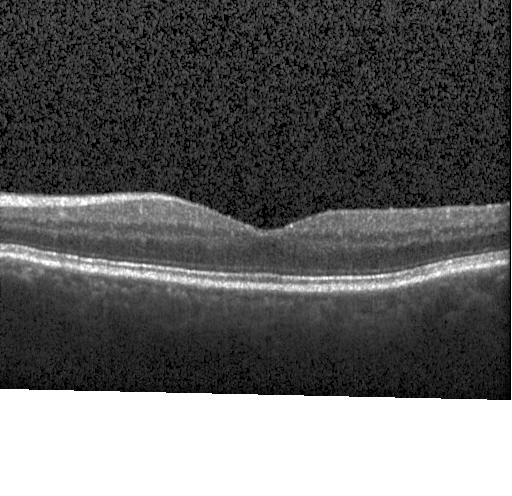 Macular scan, Heidelberg Spectralis, retinal OCT cross-section, SD-OCT
Finding: no choroidal neovascularization, no diabetic macular edema, and no drusen.